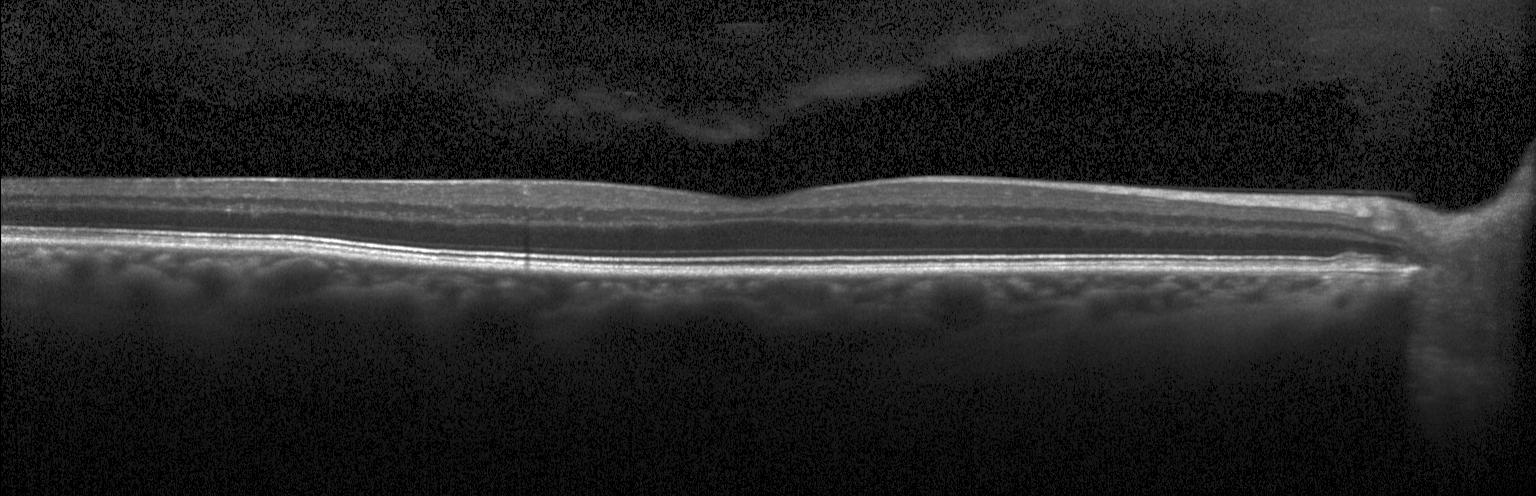
Impression: no choroidal neovascularization, no diabetic macular edema, and no drusen.